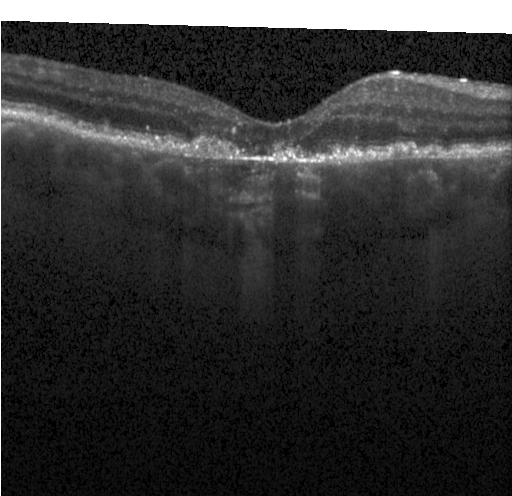
Retinal OCT cross-section
Diagnosis: choroidal neovascularization.